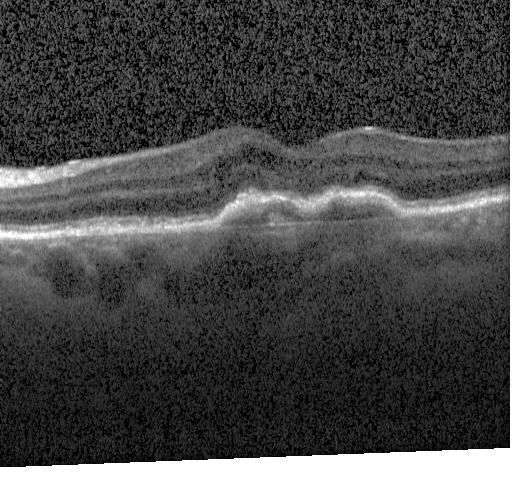
Spectral-domain OCT; OCT line scan — The scan shows a choroidal neovascular membrane.